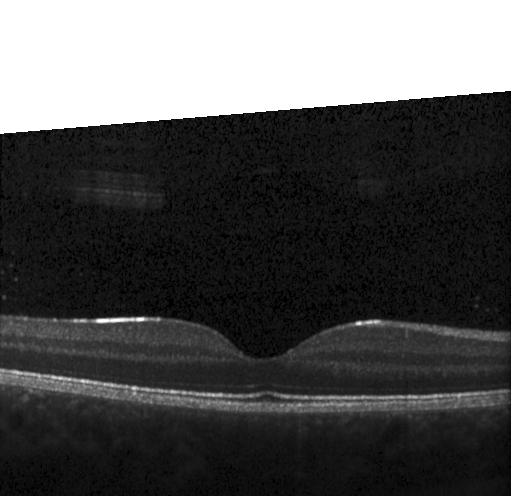 OCT line scan. The scan shows no choroidal neovascularization, diabetic macular edema, or drusen.